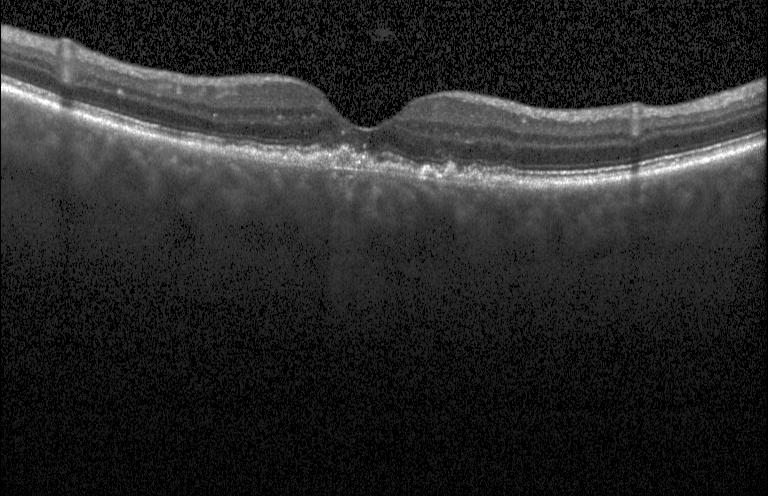
Retinal OCT B-scan · spectral-domain OCT · macular scan · acquired on a Heidelberg Spectralis. Diagnosis: a choroidal neovascular membrane.